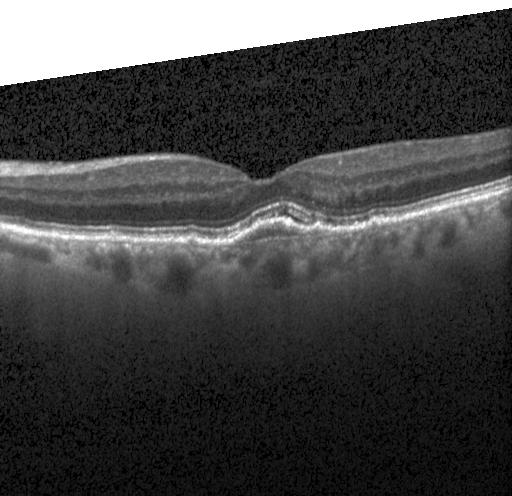

Horizontal scan through the fovea. Instrument: Heidelberg Spectralis. OCT B-scan — CNV.